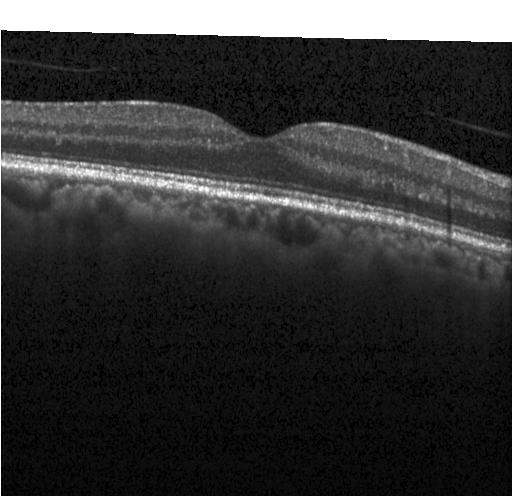 Diagnosis: no choroidal neovascularization, diabetic macular edema, or drusen.